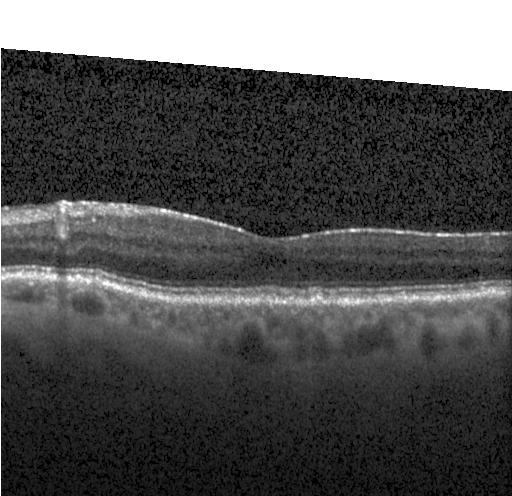

Dx: drusen.